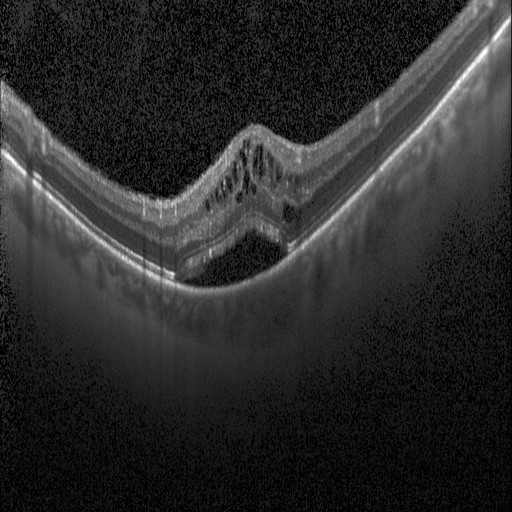 OCT B-scan showing DME.